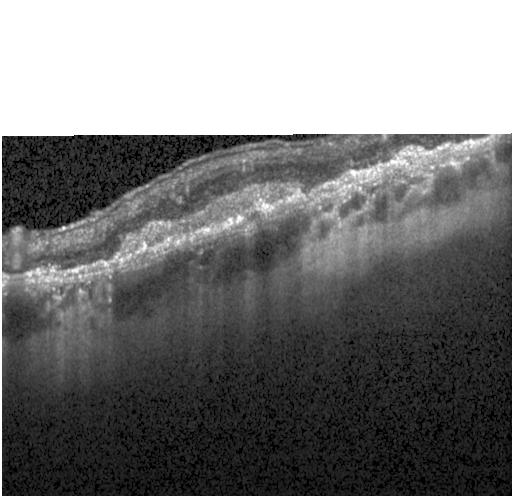 Retinal OCT B-scan; Heidelberg Spectralis OCT system; SD-OCT.
Finding: CNV.